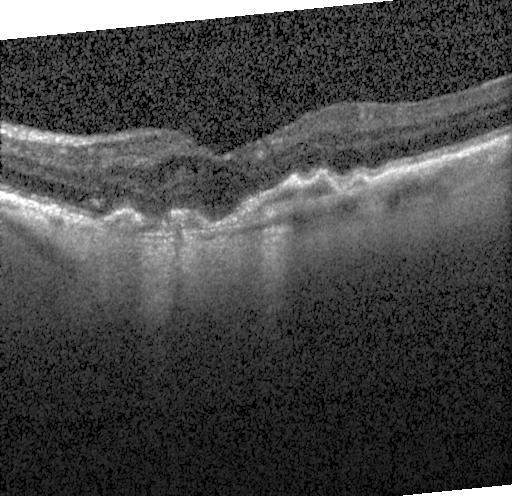
Horizontal scan through the fovea; OCT line scan; spectral-domain OCT; Heidelberg Spectralis.
Impression: choroidal neovascularization.